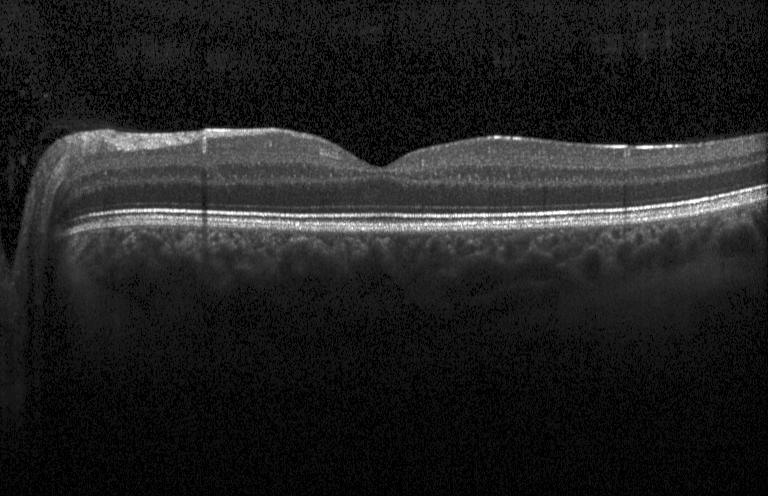

Spectral-domain OCT · acquired on a Heidelberg Spectralis · horizontal scan through the fovea · OCT line scan — The scan shows no evidence of choroidal neovascularization, diabetic macular edema, or drusen.